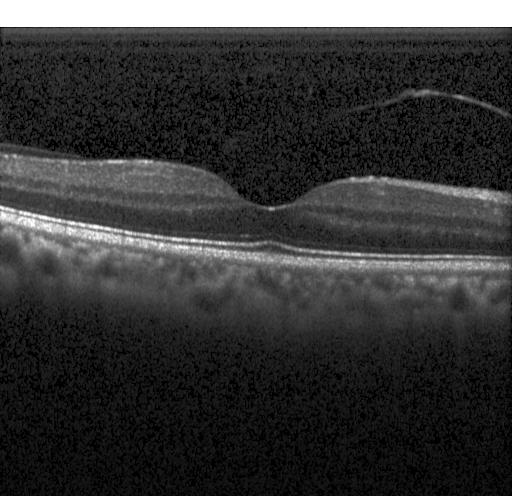 Macular scan. Optical coherence tomography scan. Instrument: Heidelberg Spectralis. Spectral-domain optical coherence tomography. OCT finding: no evidence of choroidal neovascularization, diabetic macular edema, or drusen.